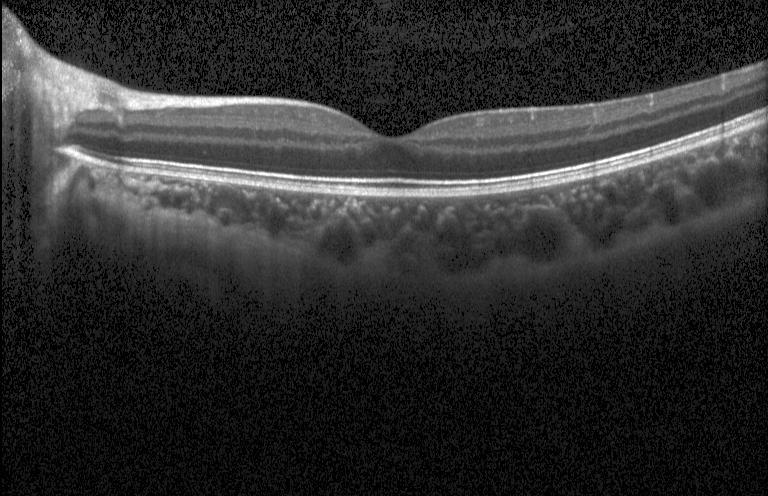

Spectral-domain OCT, acquired on a Heidelberg Spectralis, retinal OCT cross-section
Diagnosis: no choroidal neovascularization, diabetic macular edema, or drusen.